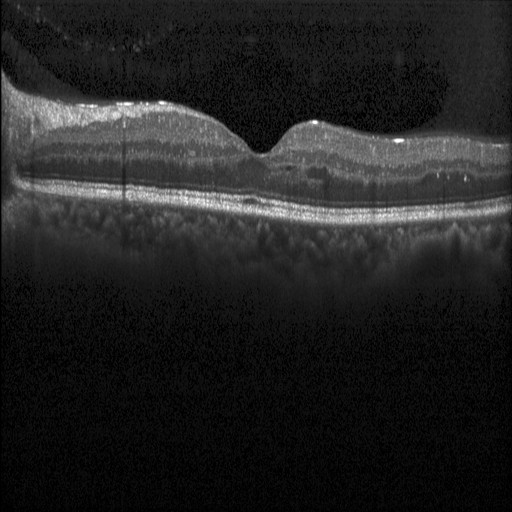 Centered on the fovea; optical coherence tomography B-scan; spectral-domain OCT.
DME.